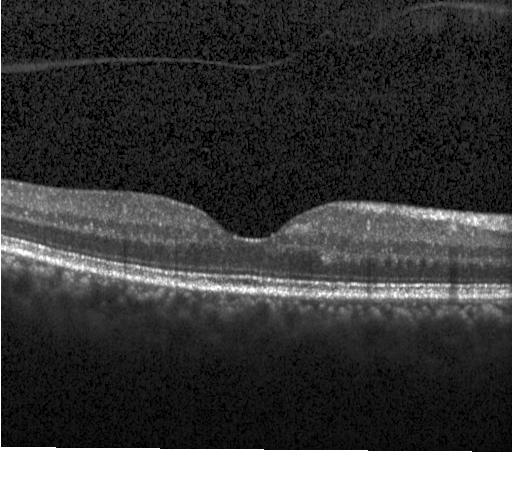

Diagnosis: no CNV, DME, or drusen.